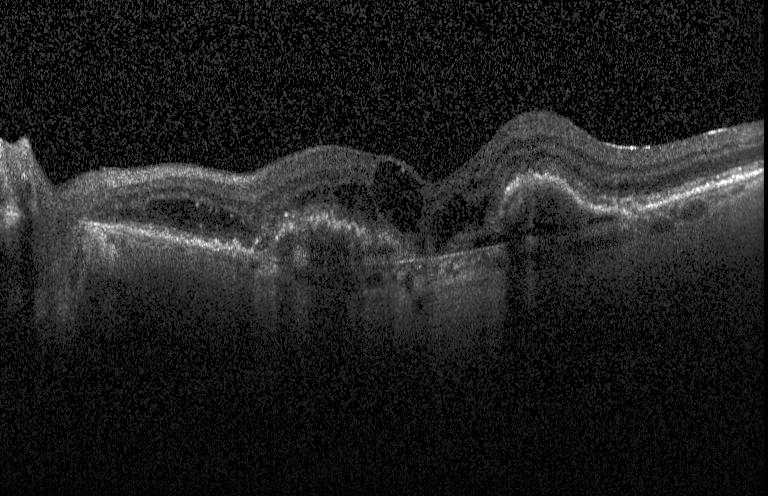 SD-OCT. OCT line scan.
Impression: choroidal neovascularization (CNV).